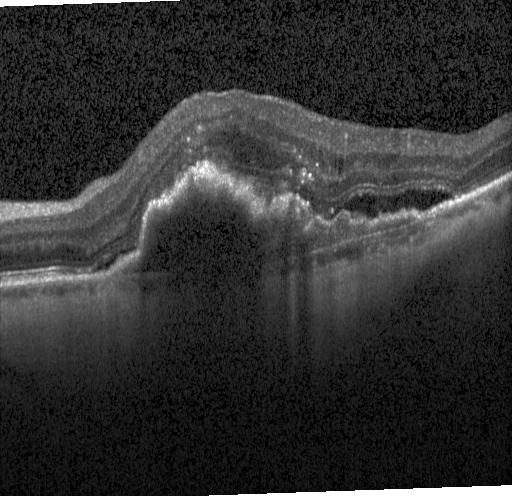 Heidelberg Spectralis OCT system · optical coherence tomography B-scan.
Diagnosis: choroidal neovascularization (CNV).